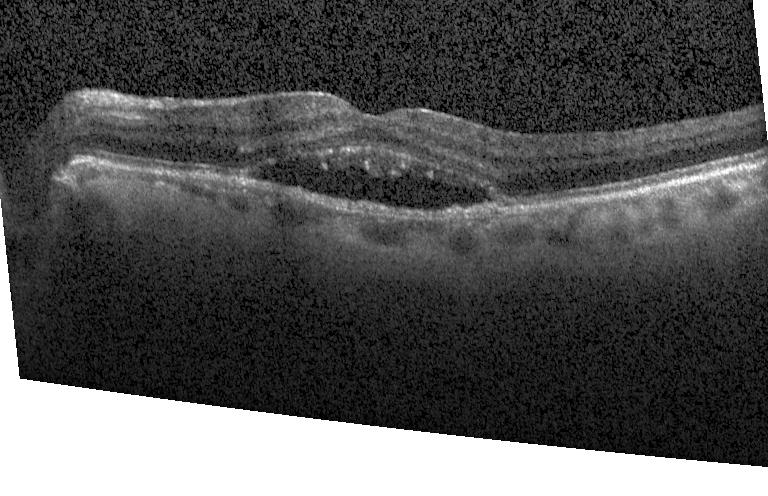 Centered on the fovea, OCT line scan, Heidelberg Spectralis
Diagnosis: choroidal neovascularization (CNV).